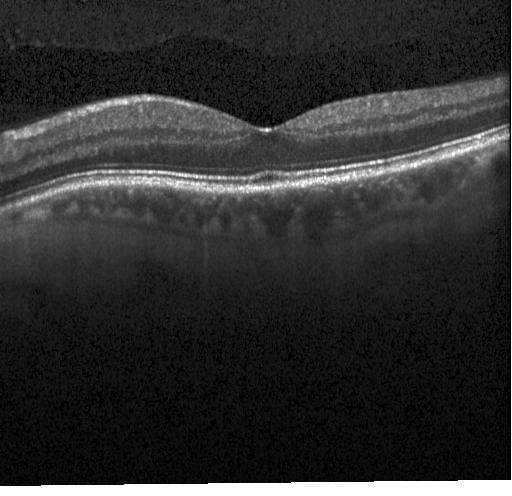 Heidelberg Spectralis OCT system · OCT B-scan · spectral-domain optical coherence tomography · horizontal scan through the fovea. Impression: no evidence of CNV, DME, or drusen.